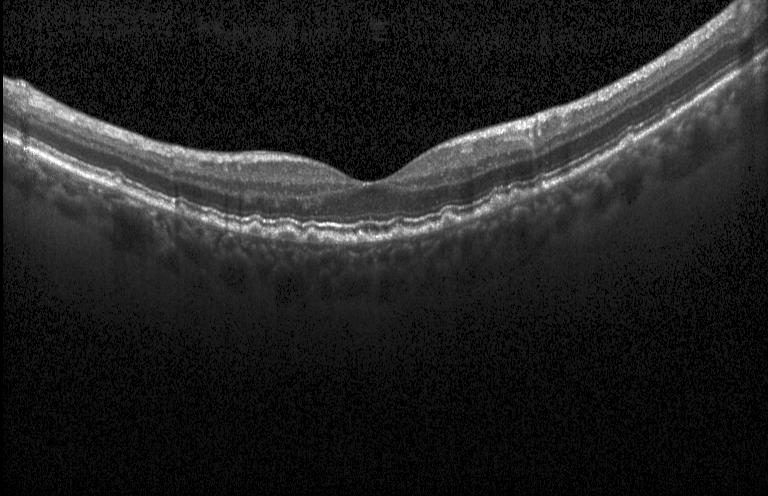

Optical coherence tomography scan.
This B-scan demonstrates multiple drusen.